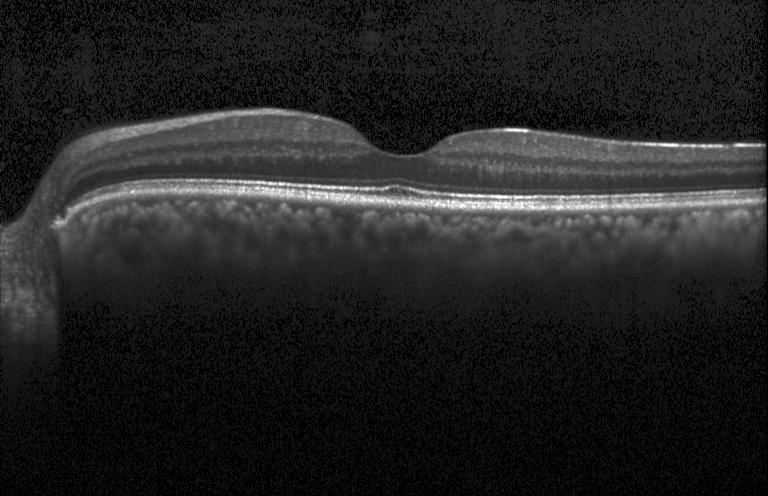 OCT line scan, centered on the fovea, SD-OCT, Heidelberg Spectralis OCT system
Diagnosis: no evidence of CNV, DME, or drusen.